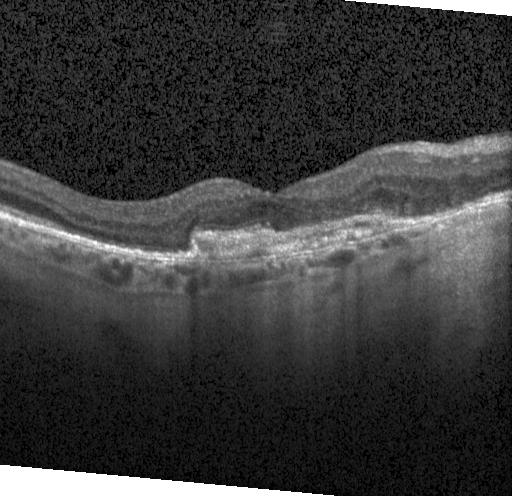 Diagnosis: choroidal neovascularization (CNV).